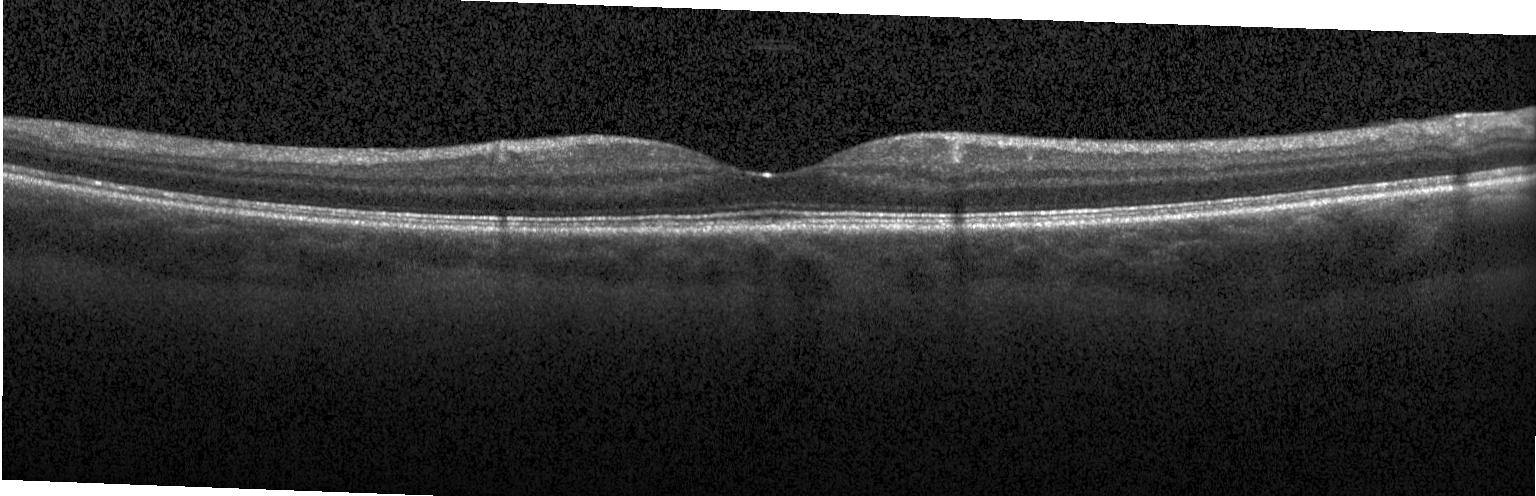 Dx: neither choroidal neovascularization, diabetic macular edema, nor drusen.